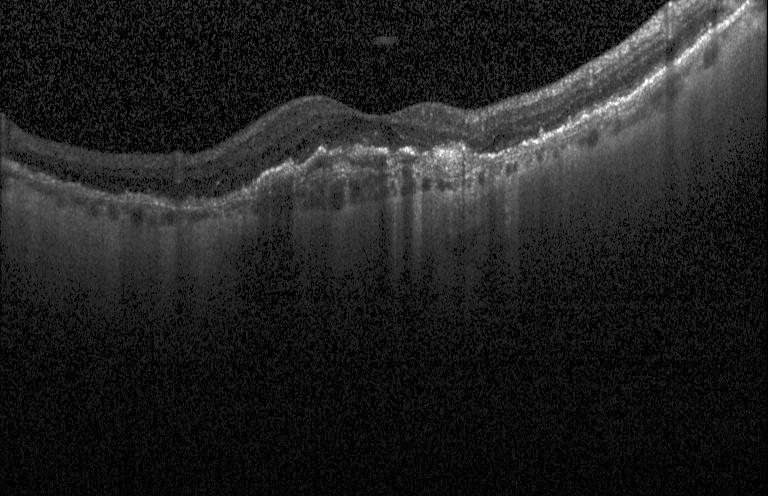 Finding: choroidal neovascularization (CNV).